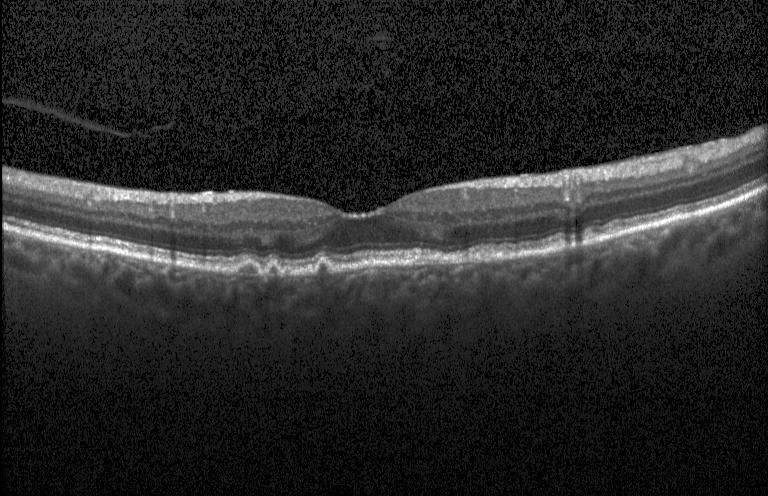

Retinal OCT cross-section — Assessment: multiple drusen.